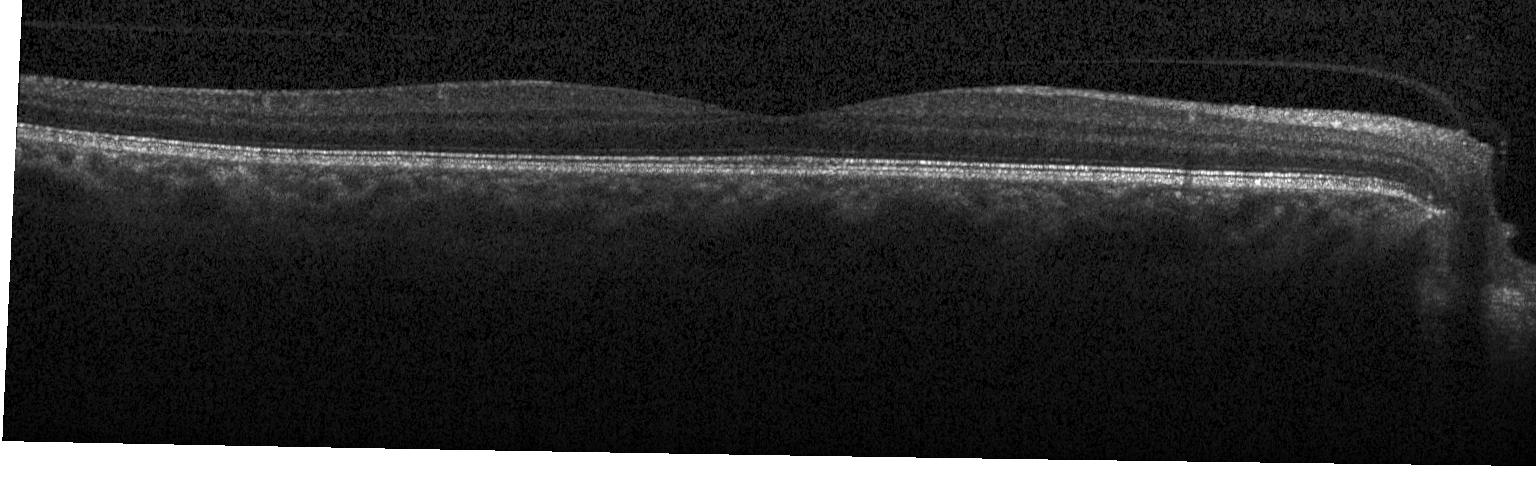 Fovea-centered. OCT line scan. Heidelberg Spectralis. Spectral-domain OCT — Finding: no evidence of choroidal neovascularization, diabetic macular edema, or drusen.